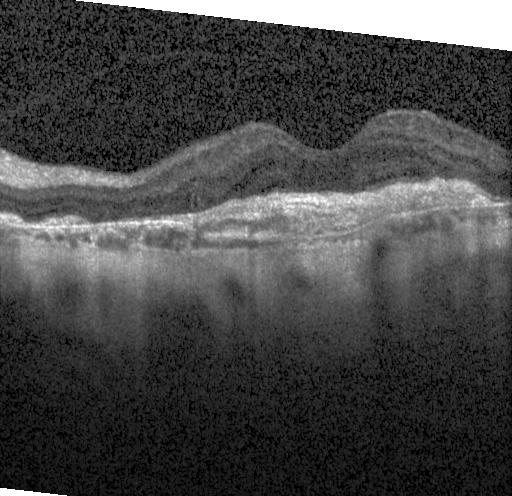 SD-OCT; Heidelberg Spectralis OCT system; retinal OCT B-scan. Impression: a choroidal neovascular membrane.